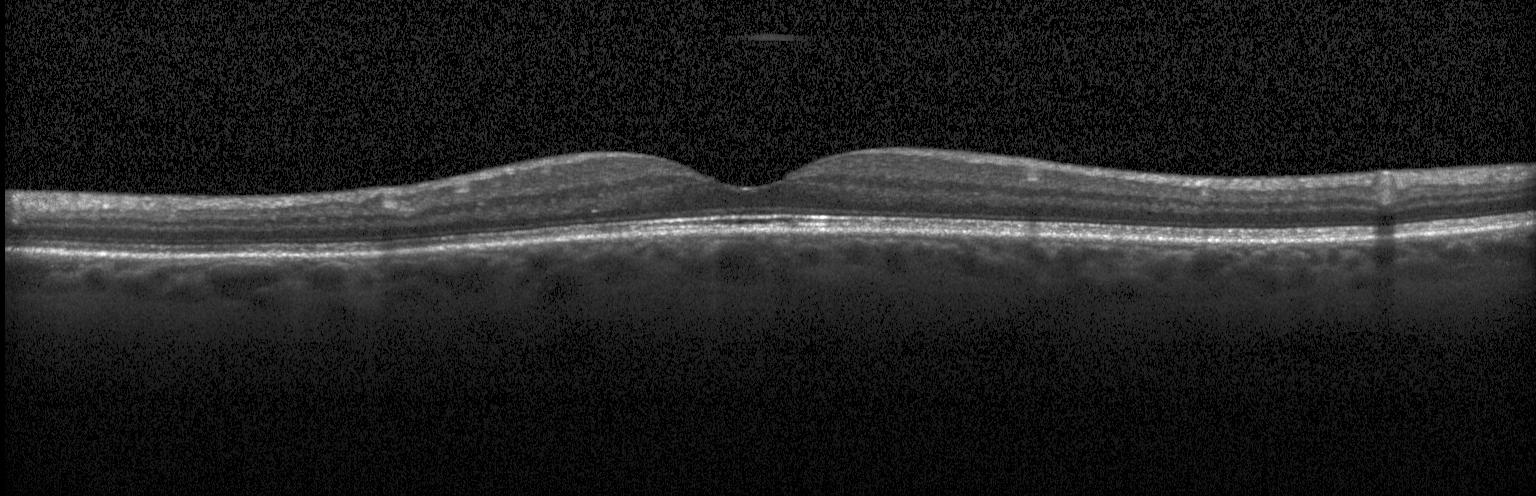

Retinal OCT cross-section.
Dx: neither choroidal neovascularization, diabetic macular edema, nor drusen.